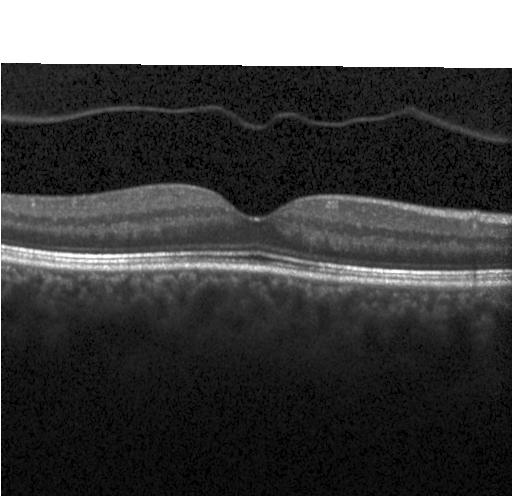

Optical coherence tomography scan; spectral-domain optical coherence tomography; Heidelberg Spectralis OCT system
Dx: no evidence of choroidal neovascularization, diabetic macular edema, or drusen.